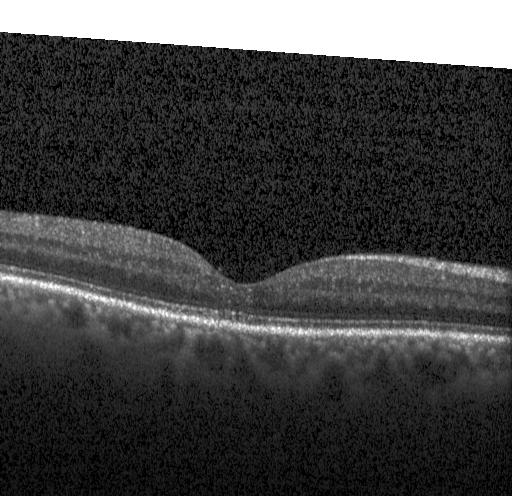
Impression: no CNV, DME, or drusen.